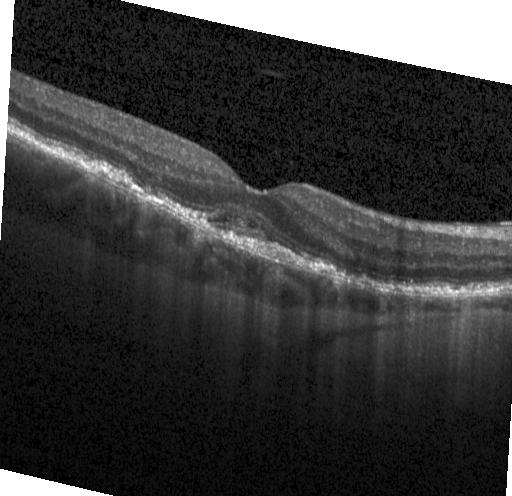

Optical coherence tomography scan. Impression: CNV.